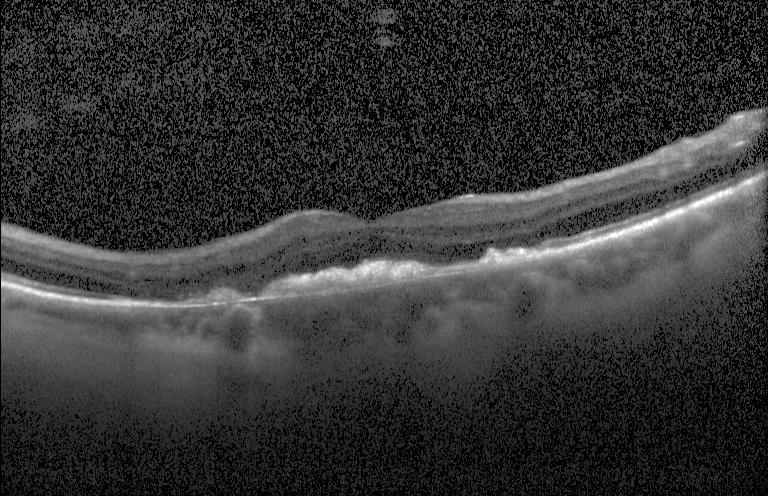
Retinal OCT cross-section showing choroidal neovascularization.